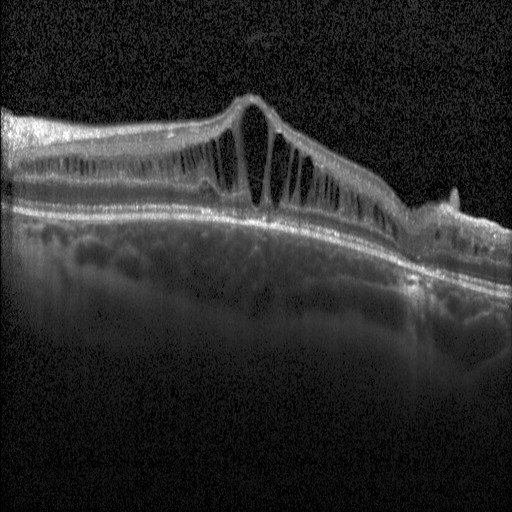 OCT finding: DME.